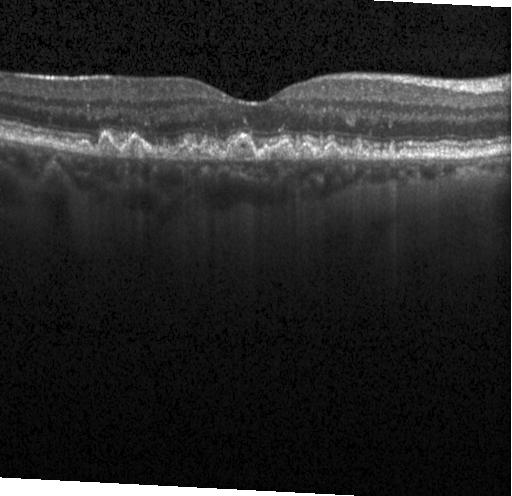 Retinal OCT cross-section. Fovea-centered. Impression: drusen.